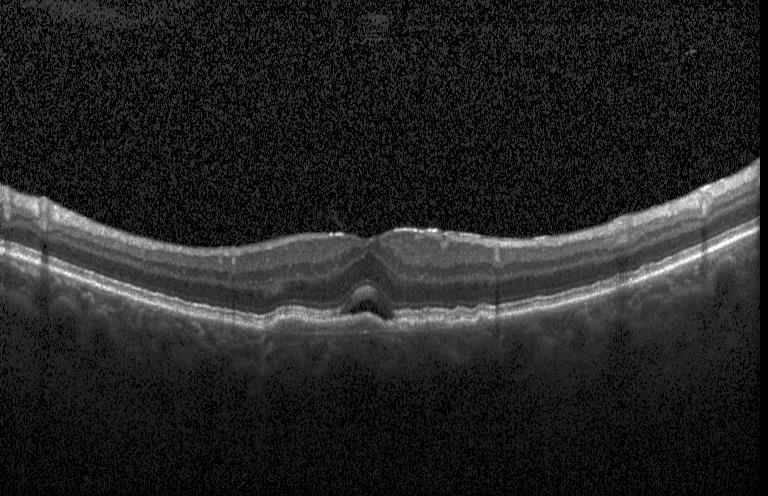

OCT B-scan. Spectral-domain optical coherence tomography. Impression: choroidal neovascularization (CNV).